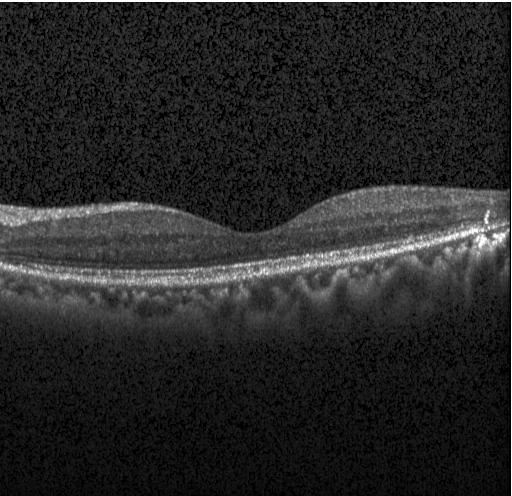 Impression: no evidence of choroidal neovascularization, diabetic macular edema, or drusen.